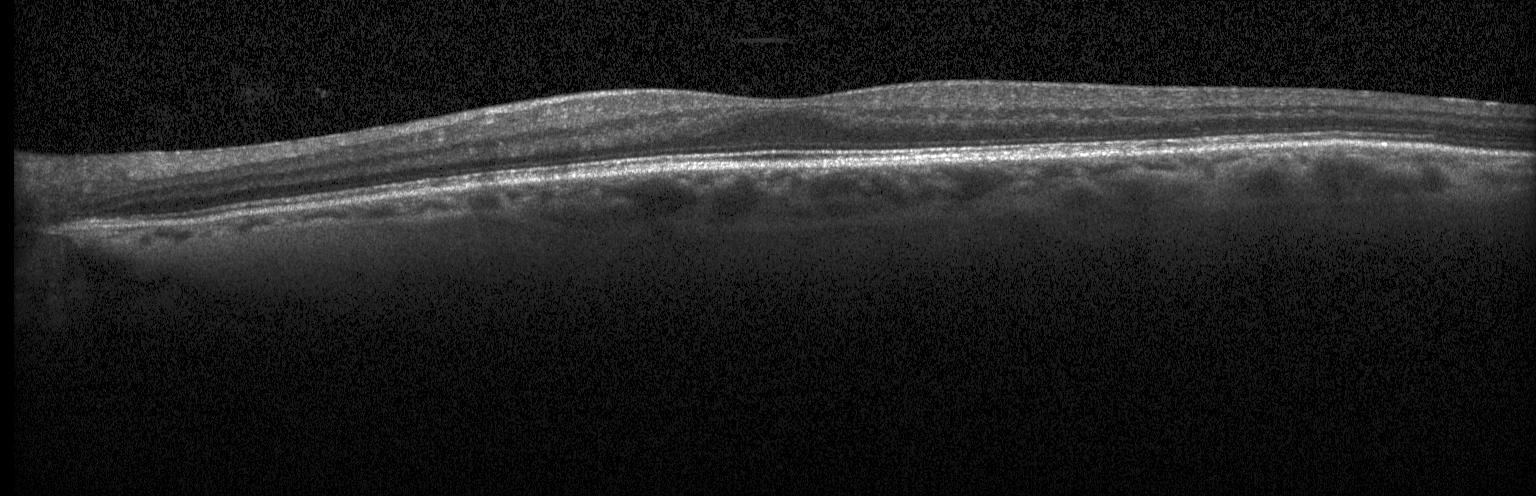

OCT B-scan, instrument: Heidelberg Spectralis. Dx: no choroidal neovascularization, no diabetic macular edema, and no drusen.